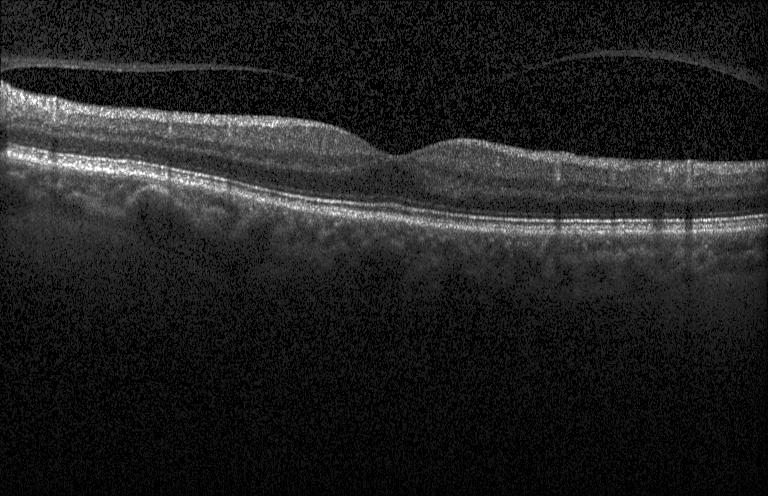

Through the macula; optical coherence tomography B-scan.
Diagnosis: no CNV, no DME, and no drusen.